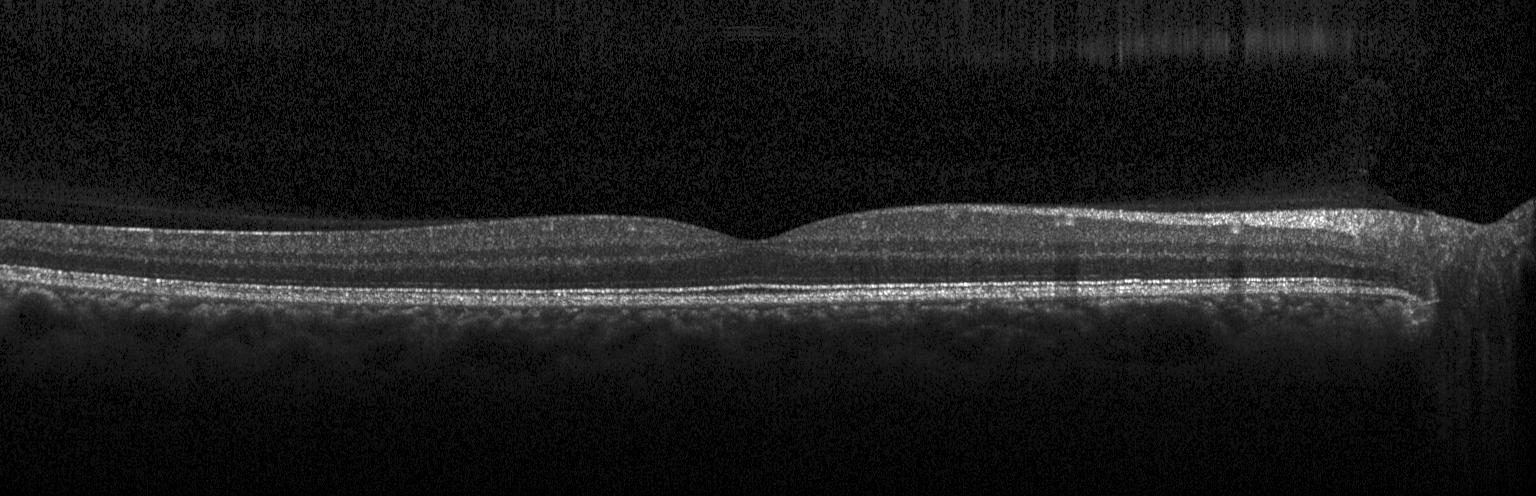

OCT scan showing no evidence of choroidal neovascularization, diabetic macular edema, or drusen.